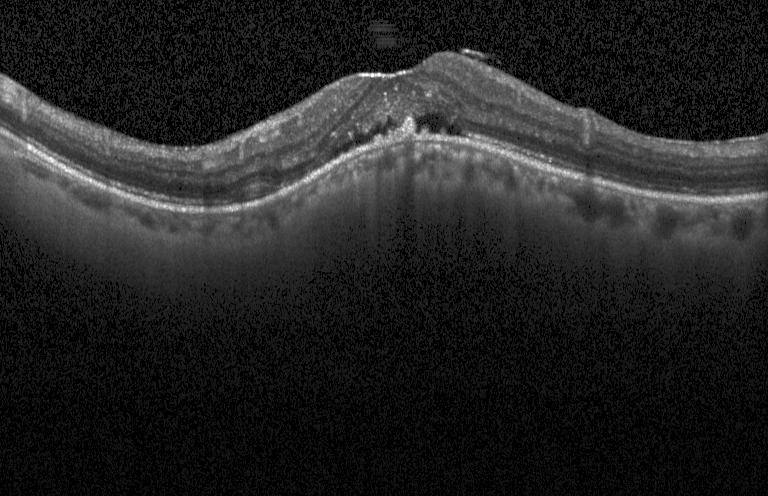 Dx: choroidal neovascularization (CNV).